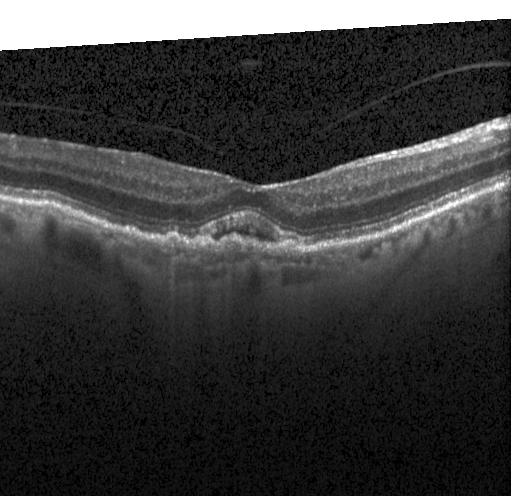 OCT finding: a choroidal neovascular membrane.